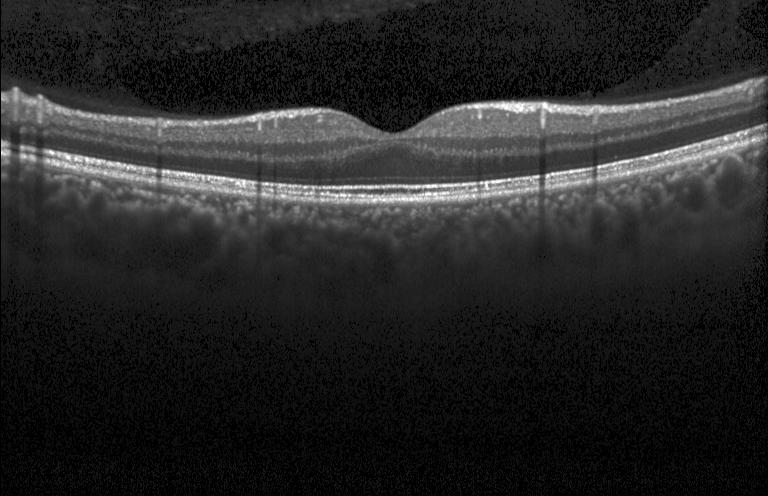
Optical coherence tomography scan
No evidence of CNV, DME, or drusen.